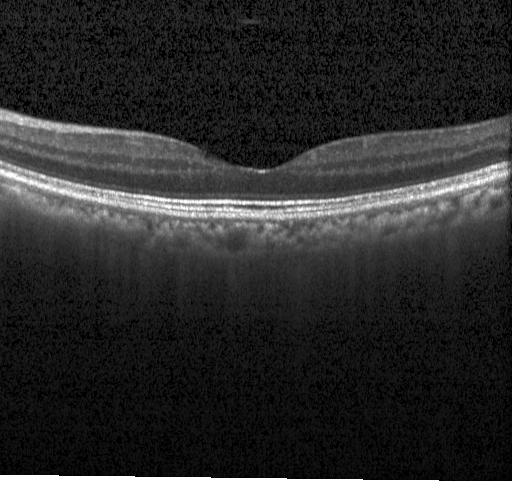

Macular OCT: no CNV, no DME, and no drusen.